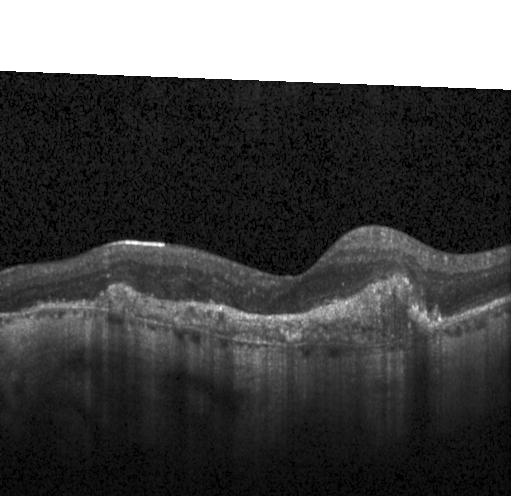 OCT line scan.
Impression: a choroidal neovascular membrane.